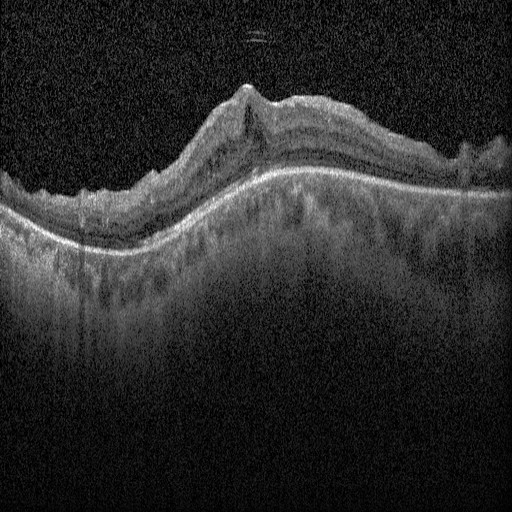

OCT line scan. Acquired on a Heidelberg Spectralis. Centered on the fovea. SD-OCT.
The scan shows diabetic macular edema (DME).